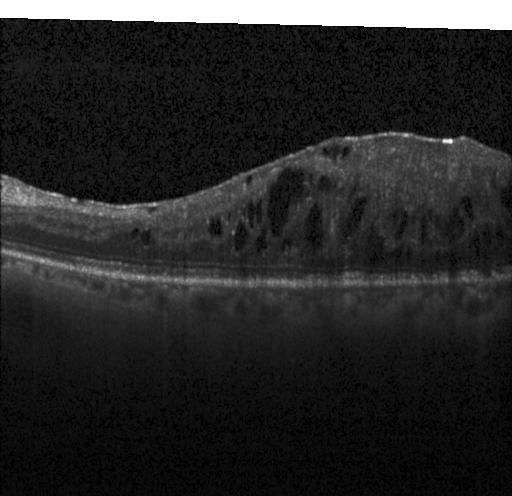

Fovea-centered. Retinal OCT B-scan. Spectral-domain OCT.
OCT finding: DME.